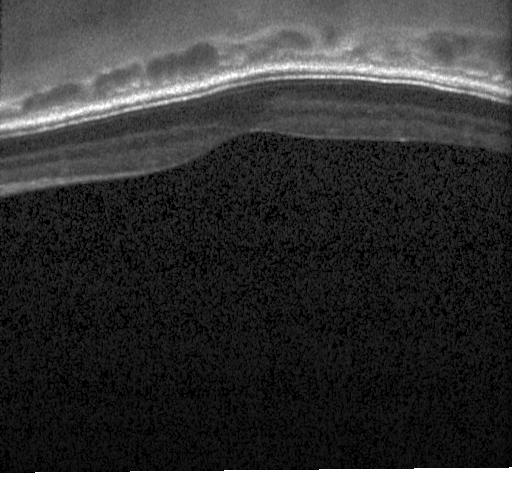
Through the macula, instrument: Heidelberg Spectralis, retinal OCT B-scan, SD-OCT
Diagnosis: neither choroidal neovascularization, diabetic macular edema, nor drusen.